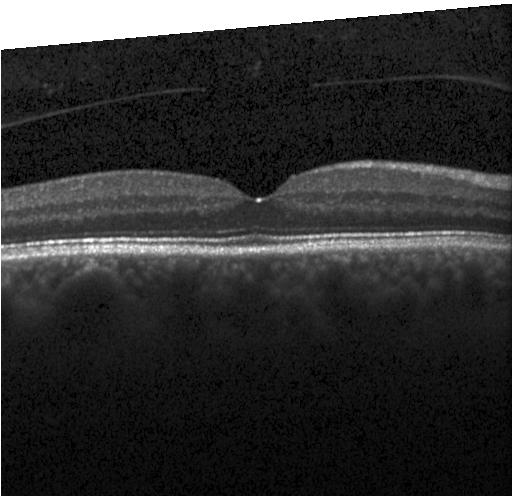 Finding: no CNV, DME, or drusen.